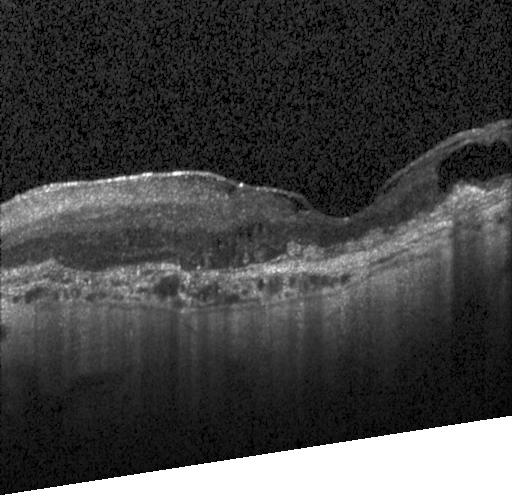

SD-OCT, acquired on a Heidelberg Spectralis, retinal OCT cross-section.
Impression: choroidal neovascularization.